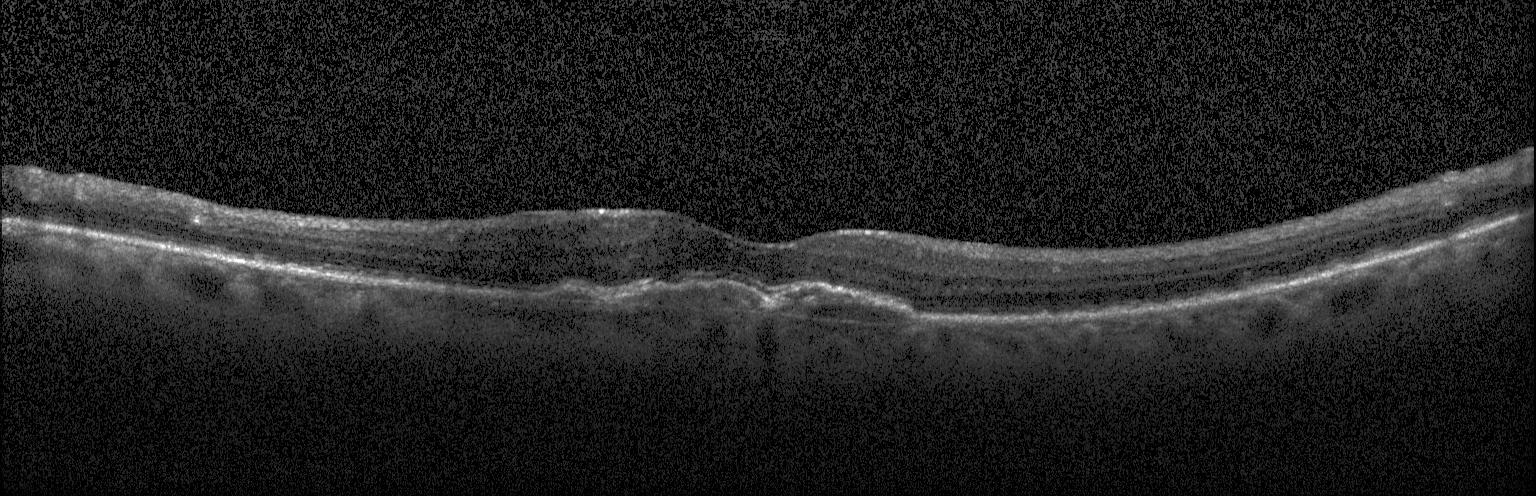
Retinal OCT cross-section showing a choroidal neovascular membrane.